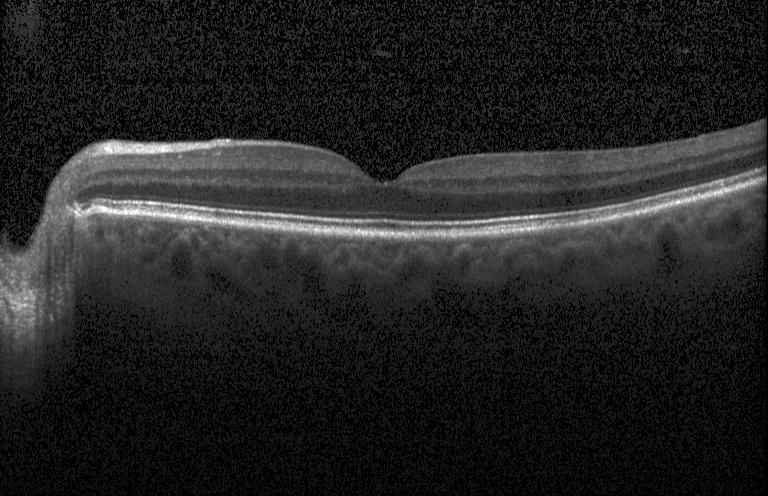
Acquired on a Heidelberg Spectralis; centered on the fovea; OCT line scan
Macular OCT: neither choroidal neovascularization, diabetic macular edema, nor drusen.